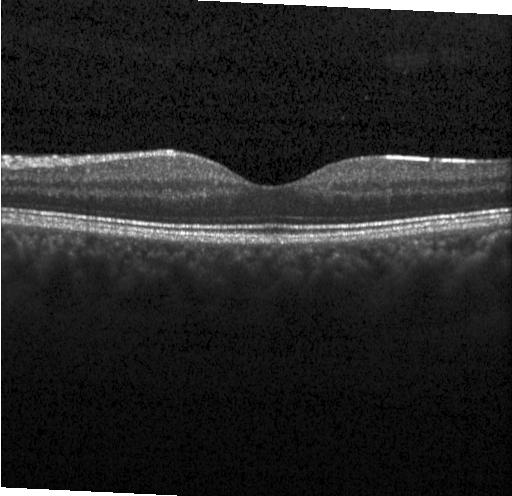

SD-OCT, retinal OCT cross-section. OCT finding: no choroidal neovascularization, no diabetic macular edema, and no drusen.